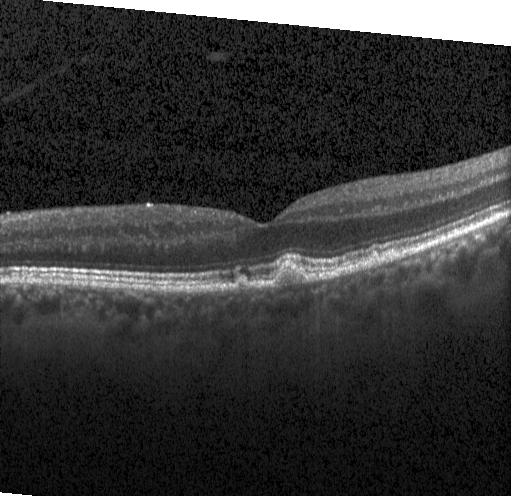 Centered on the fovea; acquired on a Heidelberg Spectralis; SD-OCT; retinal OCT cross-section — Diagnosis: multiple drusen.